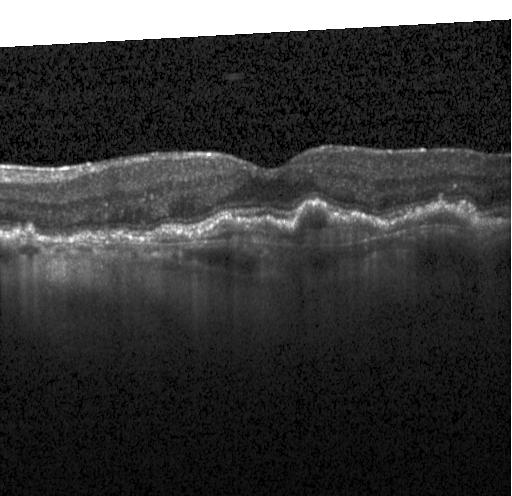 Spectral-domain OCT. Retinal OCT B-scan — Diagnosis: a choroidal neovascular membrane.